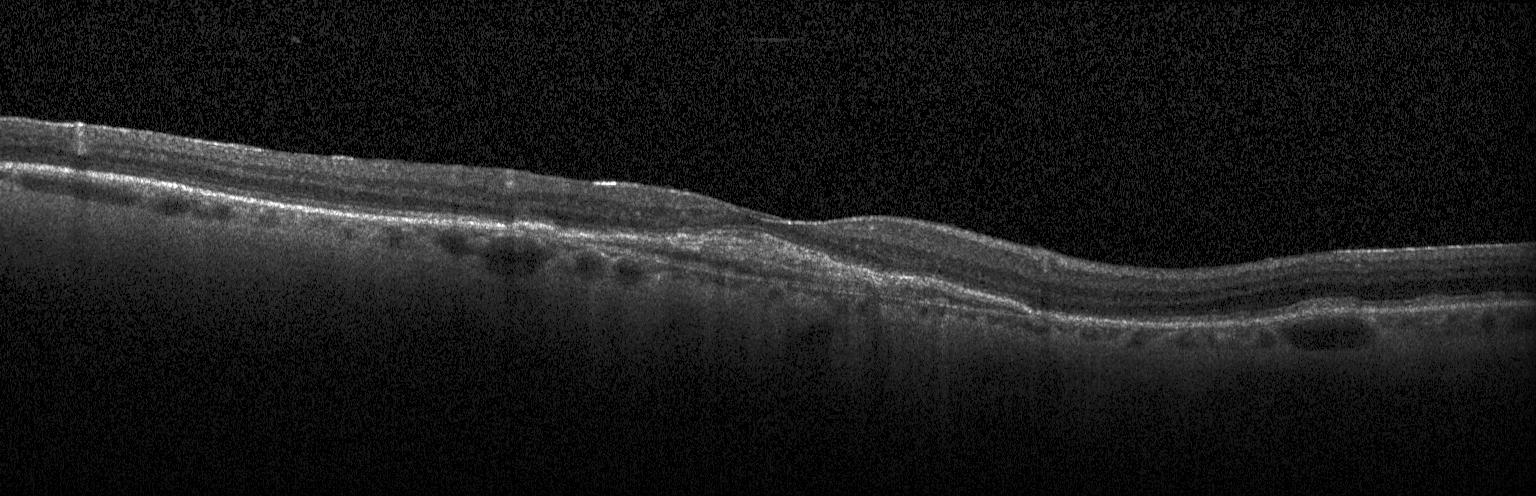
Choroidal neovascularization (CNV).